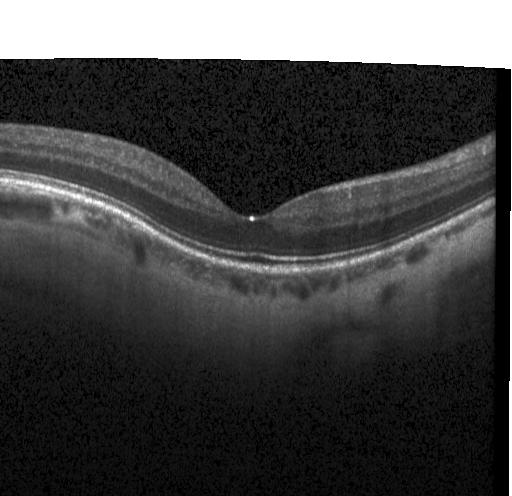
OCT B-scan; spectral-domain optical coherence tomography
Macular OCT: no CNV, no DME, and no drusen.